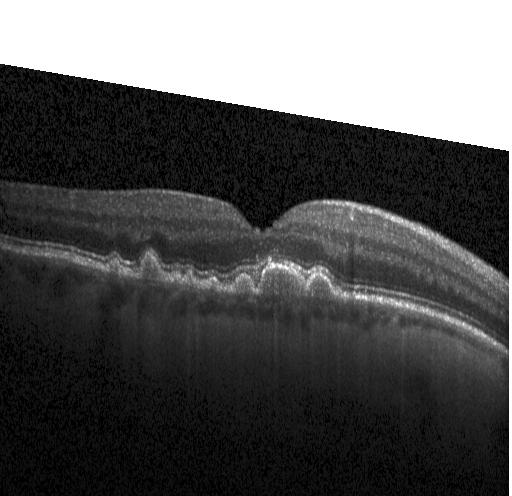

Spectral-domain OCT, horizontal scan through the fovea, acquired on a Heidelberg Spectralis, OCT line scan — The scan shows drusen.